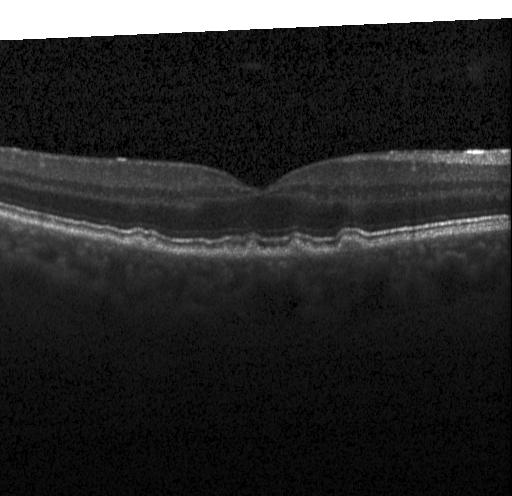 Centered on the fovea. Retinal OCT cross-section — Impression: drusen.